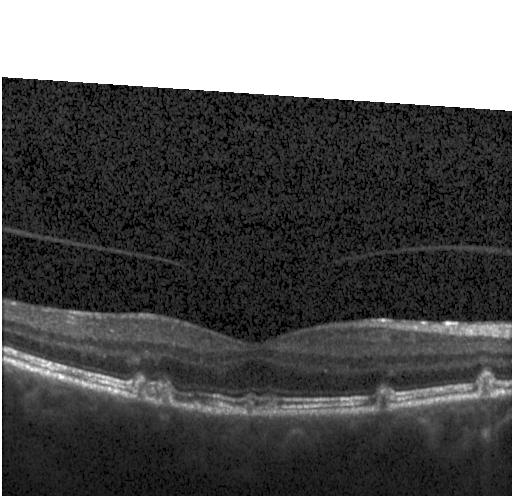

Retinal OCT B-scan, instrument: Heidelberg Spectralis, fovea-centered.
Finding: drusen.